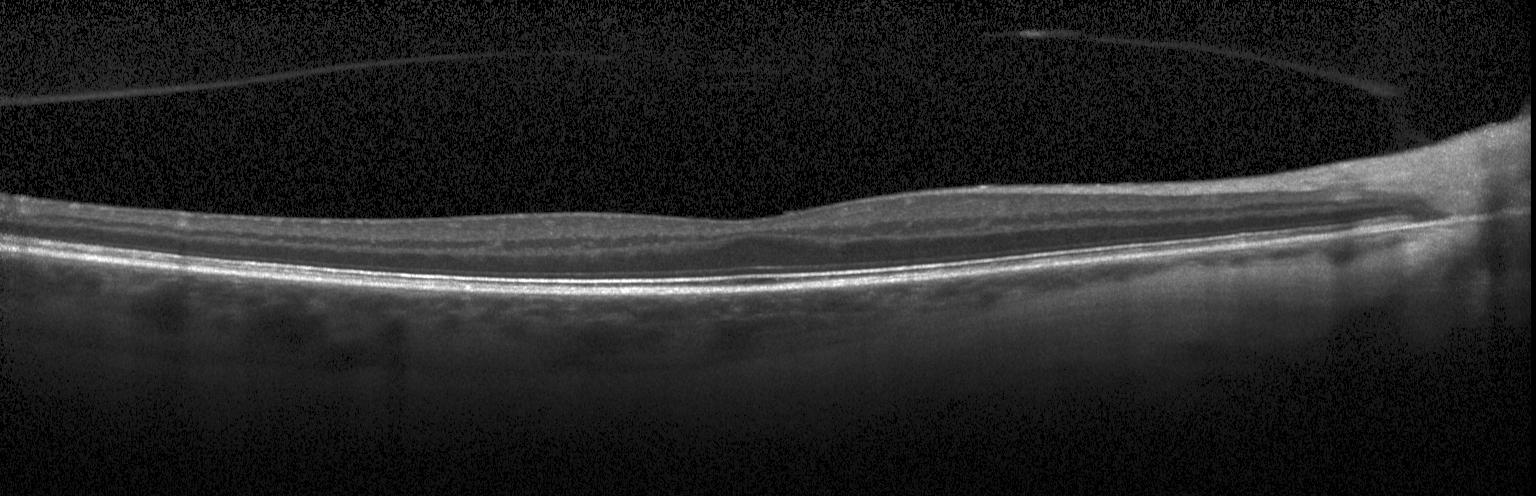 Retinal OCT B-scan — Impression: no evidence of choroidal neovascularization, diabetic macular edema, or drusen.